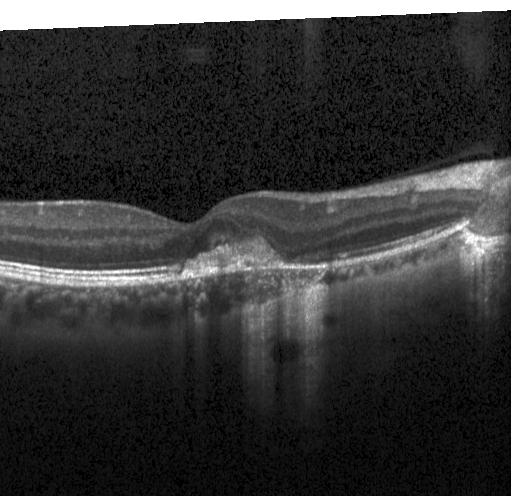 Macular OCT demonstrating a choroidal neovascular membrane.